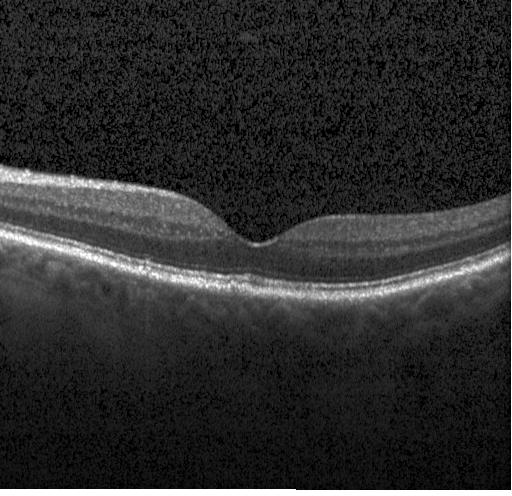

Diagnosis: no evidence of CNV, DME, or drusen.